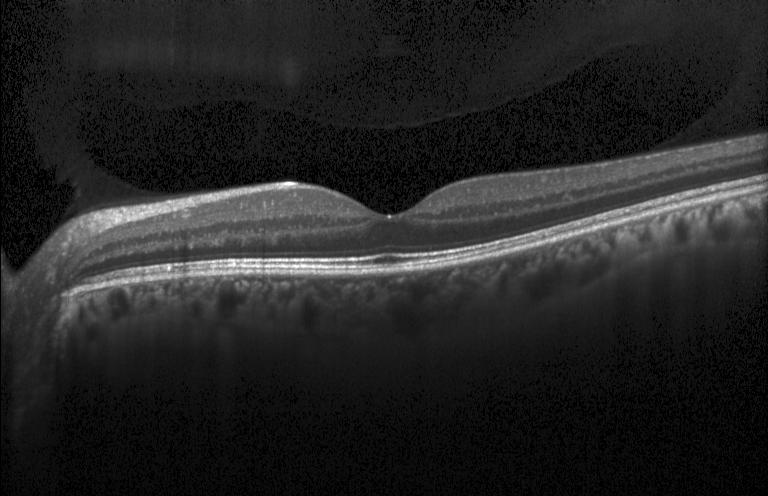

OCT line scan. Finding: no choroidal neovascularization, diabetic macular edema, or drusen.